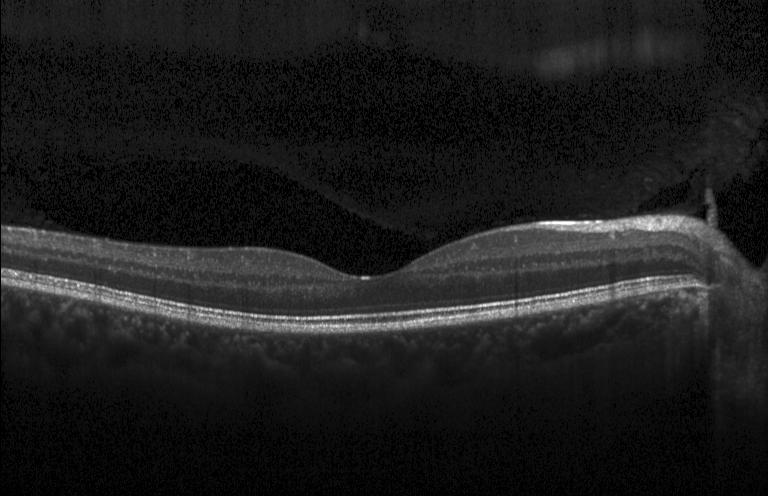
OCT B-scan; fovea-centered — OCT finding: no choroidal neovascularization, diabetic macular edema, or drusen.